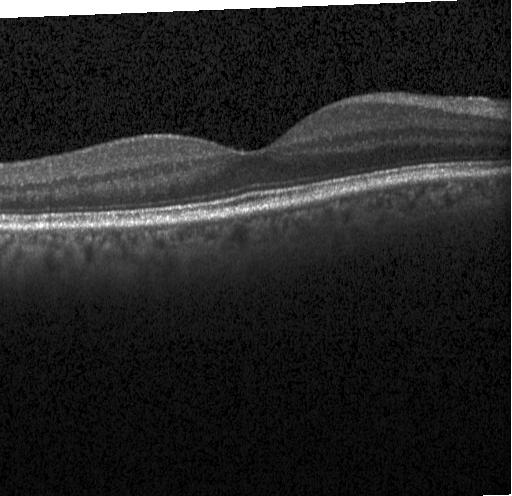
OCT B-scan showing no choroidal neovascularization, diabetic macular edema, or drusen.